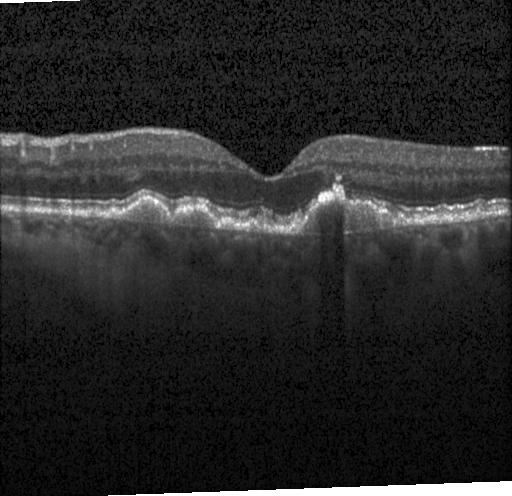
Through the macula. Spectral-domain optical coherence tomography. Optical coherence tomography B-scan. Acquired on a Heidelberg Spectralis. Assessment: multiple drusen.